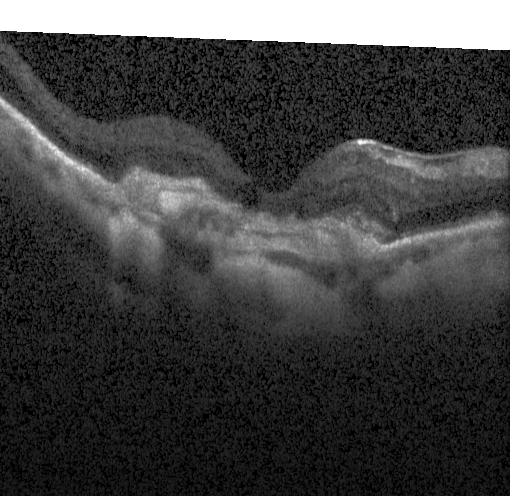 Centered on the fovea; Heidelberg Spectralis OCT system; optical coherence tomography B-scan; spectral-domain optical coherence tomography — The scan shows a choroidal neovascular membrane.